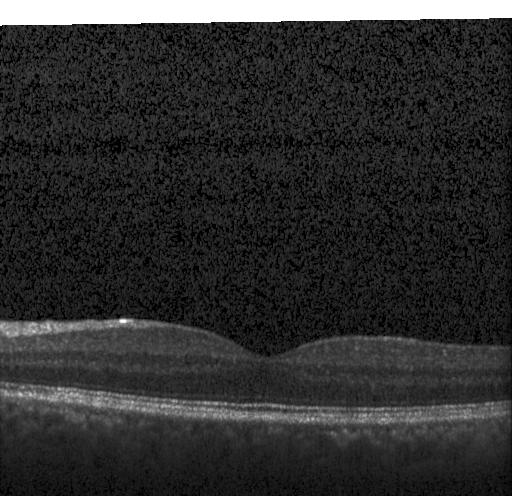 Optical coherence tomography scan; centered on the fovea. Finding: no evidence of choroidal neovascularization, diabetic macular edema, or drusen.